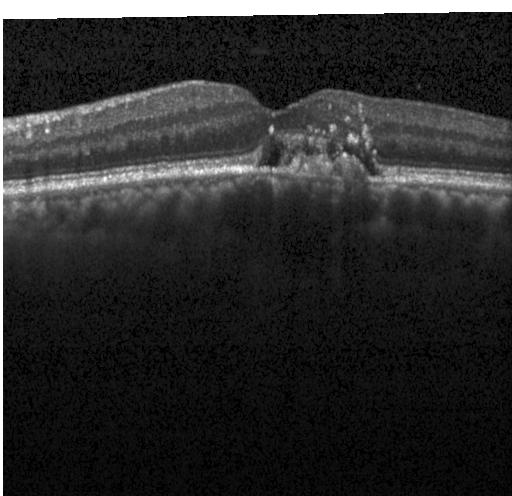
Finding: a choroidal neovascular membrane.